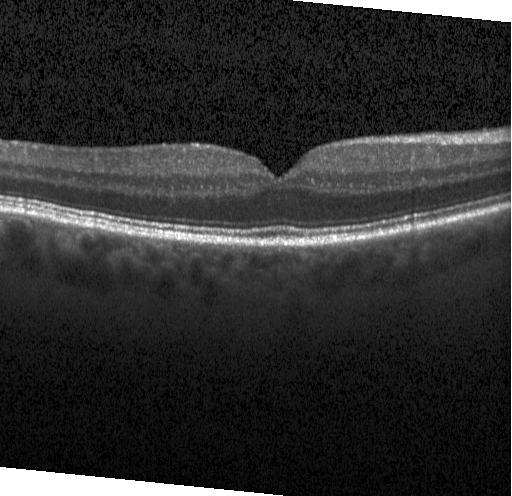 Centered on the fovea. Heidelberg Spectralis. Optical coherence tomography B-scan. Spectral-domain optical coherence tomography — Finding: neither choroidal neovascularization, diabetic macular edema, nor drusen.